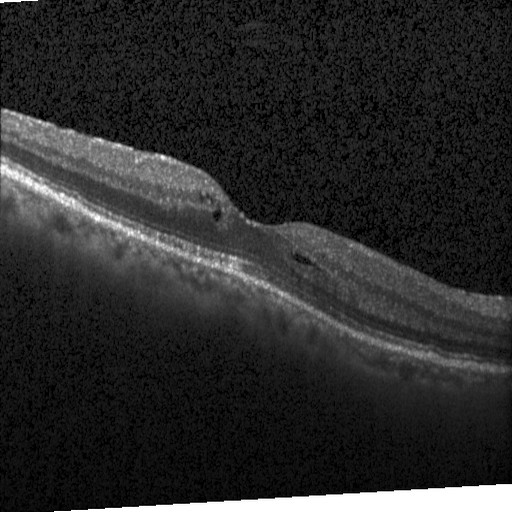

OCT B-scan showing diabetic macular edema (DME).